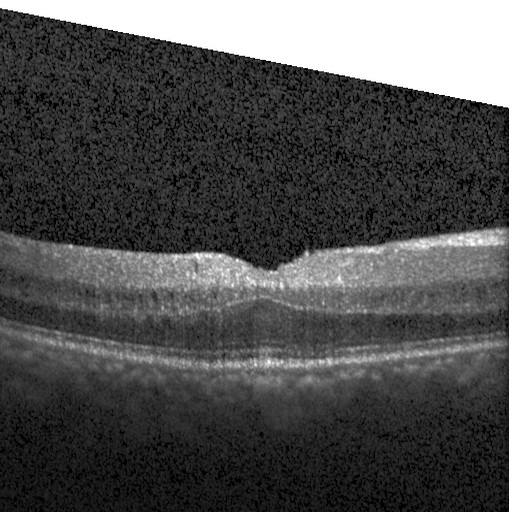 Dx: diabetic macular edema (DME).